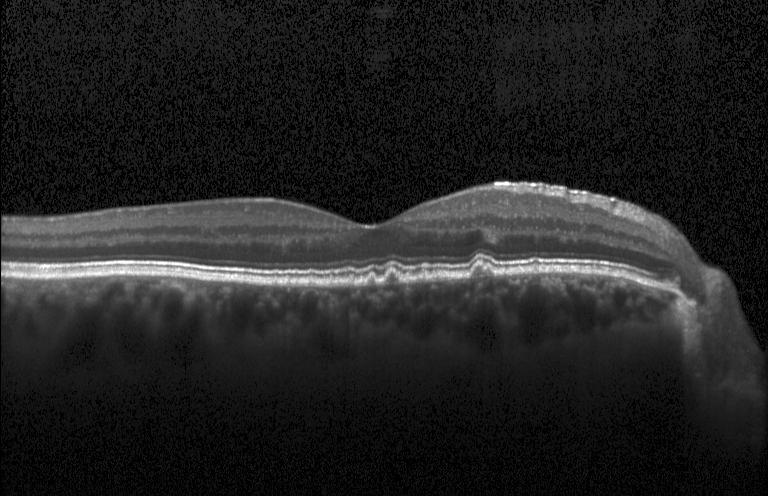

Finding: drusen.